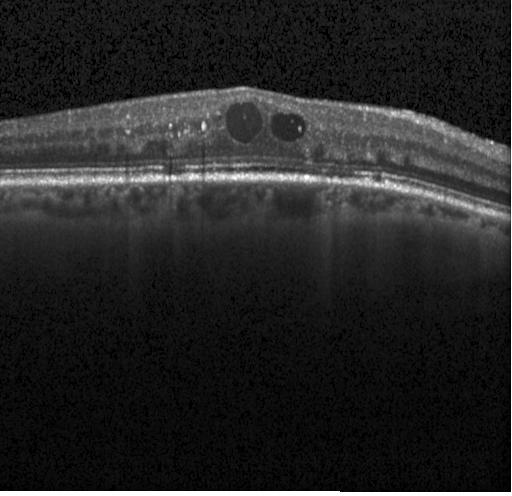

Centered on the fovea, OCT line scan — Macular OCT: DME.